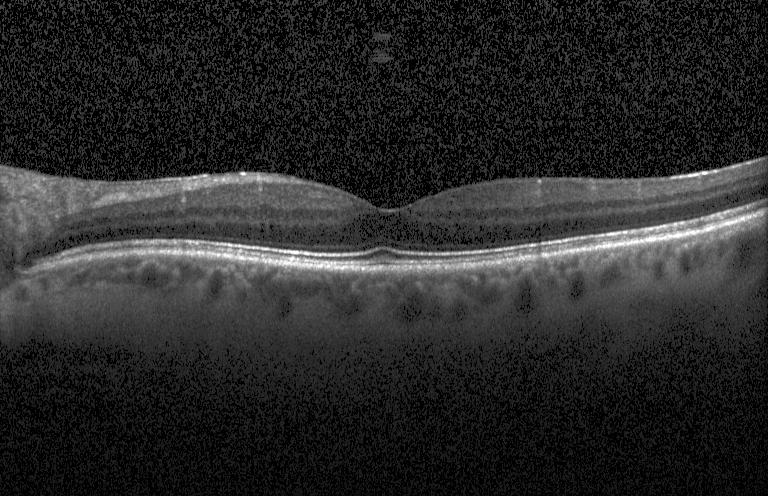
OCT line scan. Impression: no choroidal neovascularization, no diabetic macular edema, and no drusen.